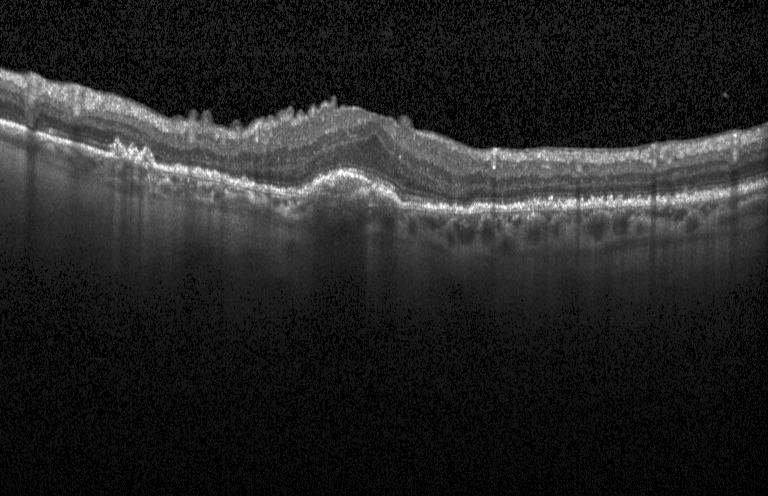

Retinal OCT B-scan.
Finding: a choroidal neovascular membrane.